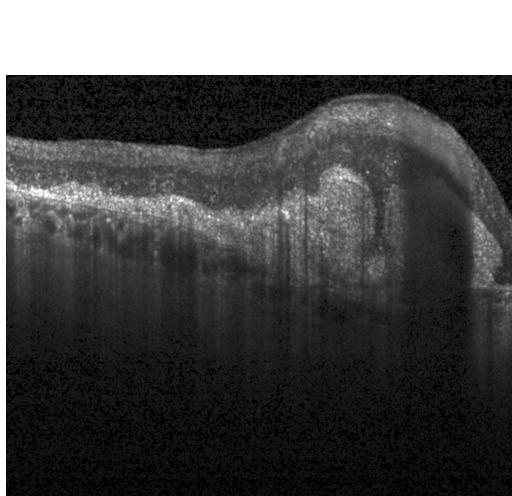 Finding: a choroidal neovascular membrane.